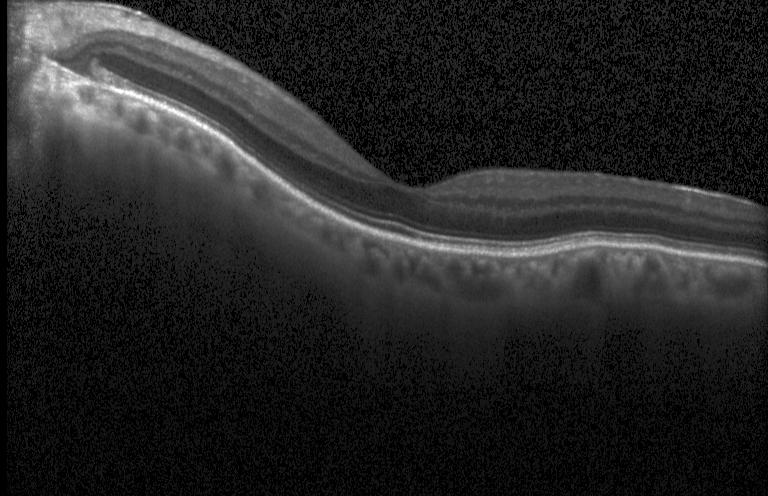

Retinal OCT cross-section showing no choroidal neovascularization, no diabetic macular edema, and no drusen.